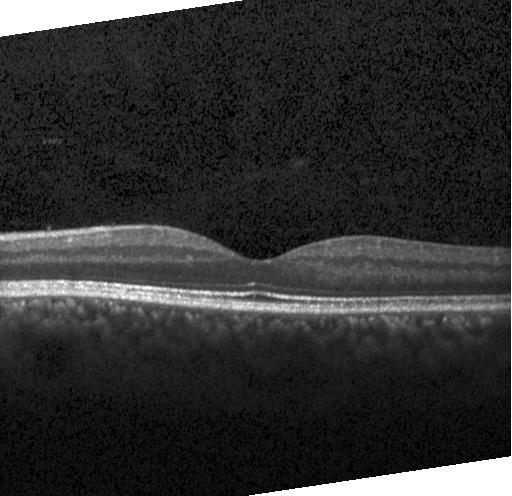

Retinal OCT cross-section; through the macula. OCT finding: neither choroidal neovascularization, diabetic macular edema, nor drusen.